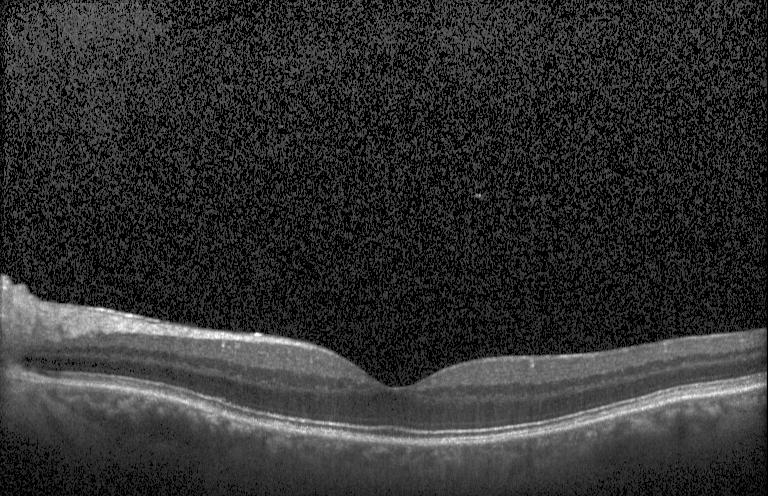
Through the macula; OCT line scan — Impression: neither choroidal neovascularization, diabetic macular edema, nor drusen.